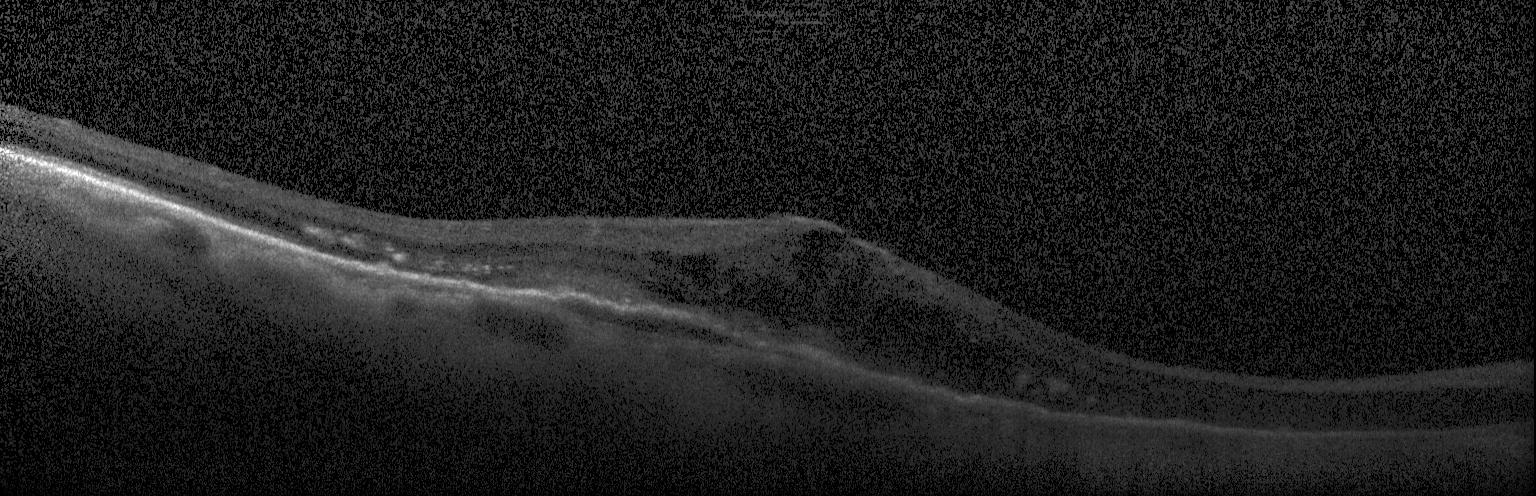 Finding: a choroidal neovascular membrane.